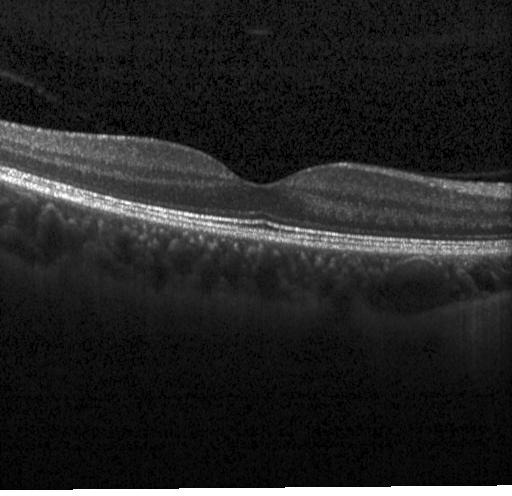
Optical coherence tomography B-scan
Impression: no evidence of choroidal neovascularization, diabetic macular edema, or drusen.